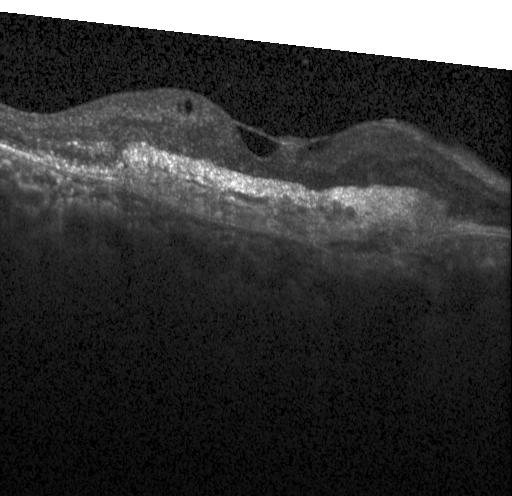 Fovea-centered. SD-OCT. OCT line scan. Dx: choroidal neovascularization (CNV).